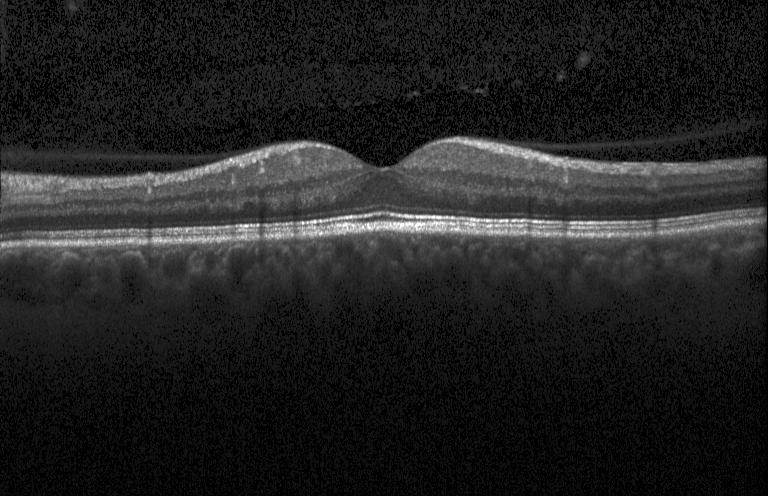 Macular OCT demonstrating no choroidal neovascularization, no diabetic macular edema, and no drusen.